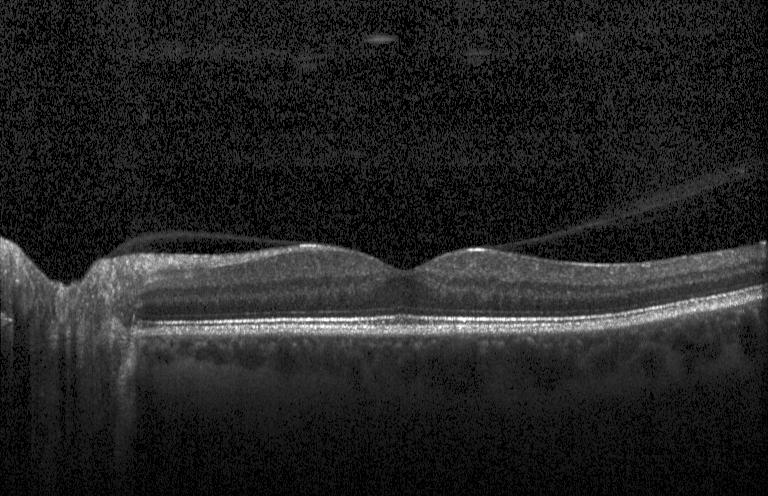 Spectral-domain optical coherence tomography · through the macula · retinal OCT B-scan · Heidelberg Spectralis OCT system. Finding: no evidence of choroidal neovascularization, diabetic macular edema, or drusen.